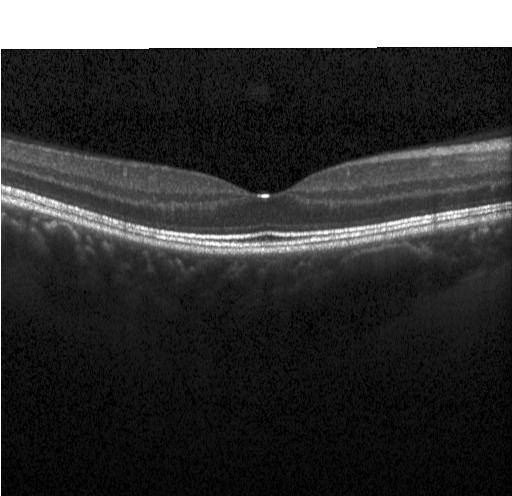 OCT line scan.
No CNV, DME, or drusen.